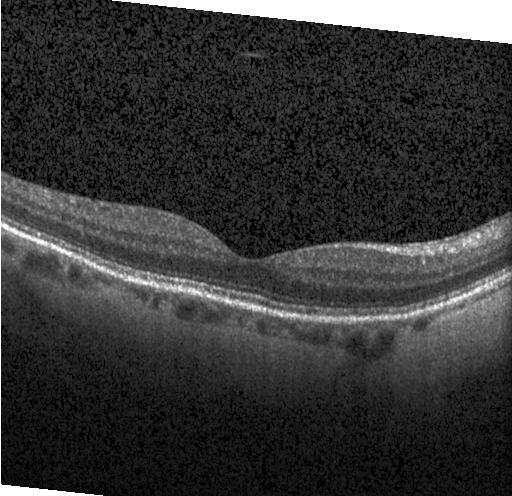
OCT B-scan.
Finding: no choroidal neovascularization, diabetic macular edema, or drusen.